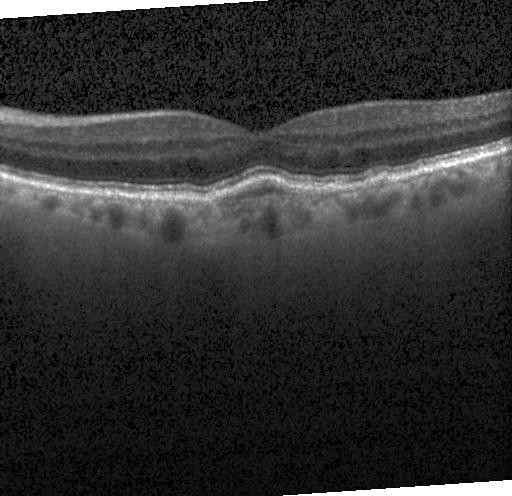
OCT line scan. SD-OCT. Fovea-centered. Instrument: Heidelberg Spectralis.
Macular OCT: a choroidal neovascular membrane.